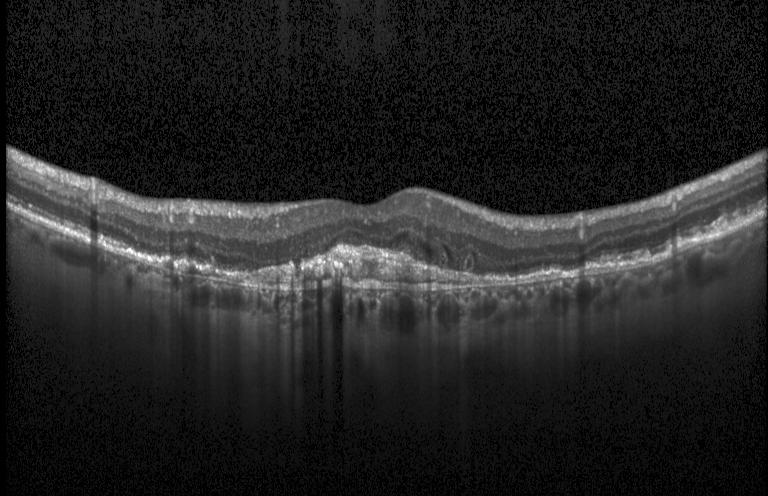 Spectral-domain optical coherence tomography; retinal OCT cross-section. Choroidal neovascularization (CNV).